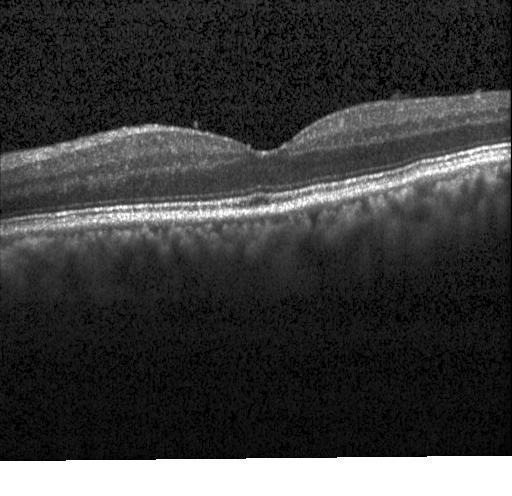

OCT line scan — Finding: no CNV, no DME, and no drusen.